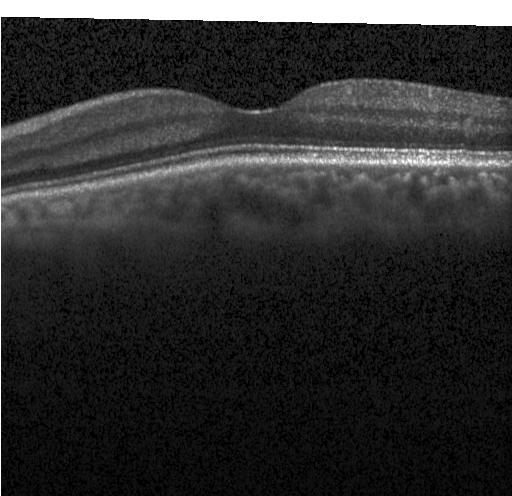 Optical coherence tomography scan — Finding: neither choroidal neovascularization, diabetic macular edema, nor drusen.